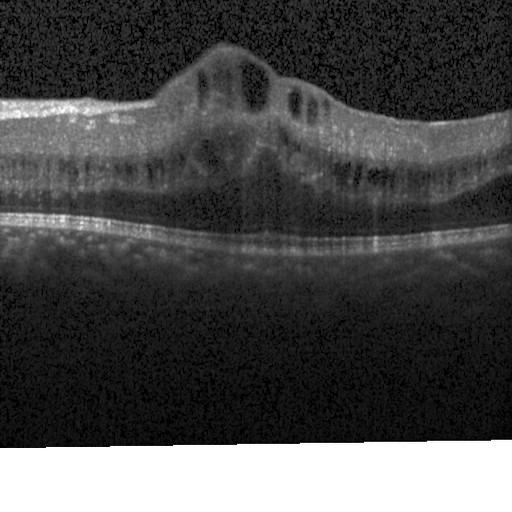
Spectral-domain optical coherence tomography; optical coherence tomography B-scan.
Diabetic macular edema.